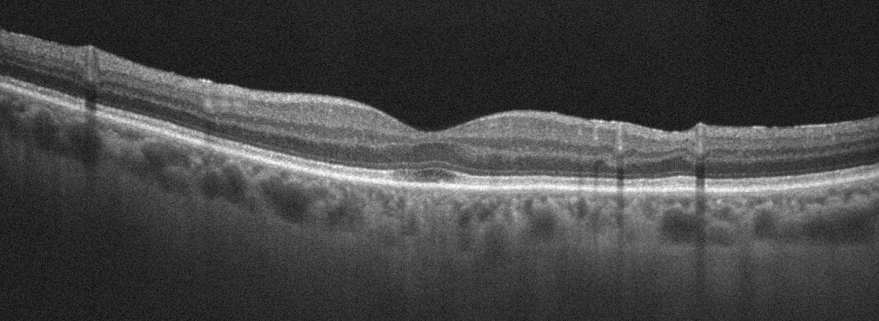 Impression: age-related macular degeneration.